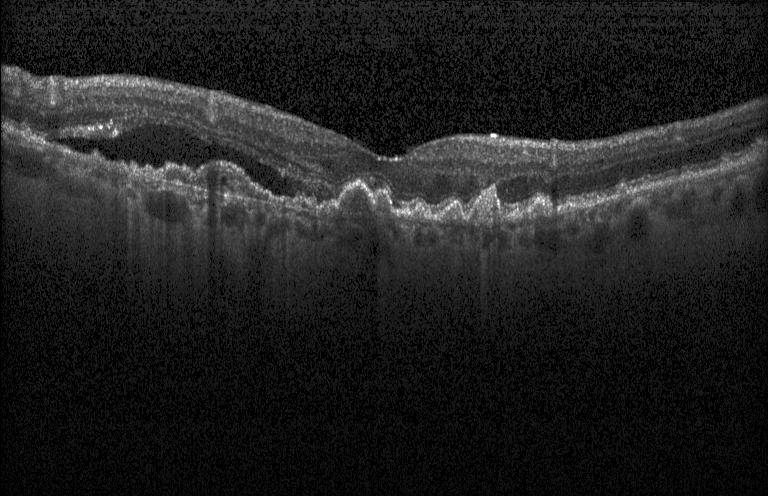 Centered on the fovea. Optical coherence tomography scan
This B-scan demonstrates a choroidal neovascular membrane.